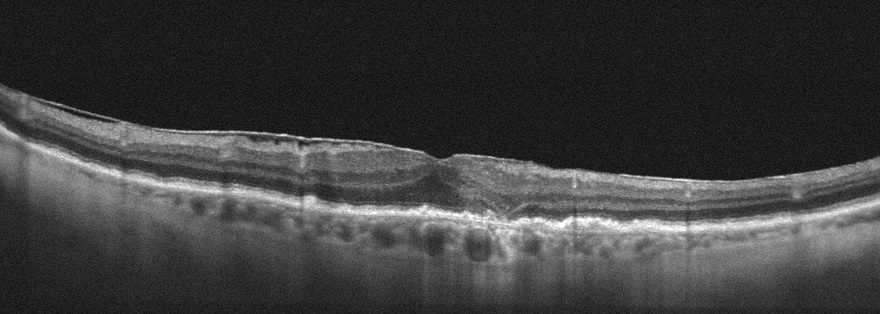
OCT scan showing ERM.